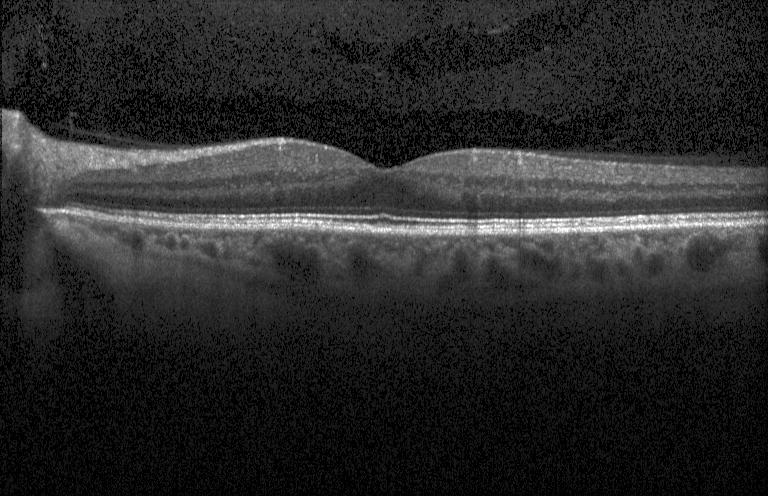 Retinal OCT cross-section showing neither CNV, DME, nor drusen.